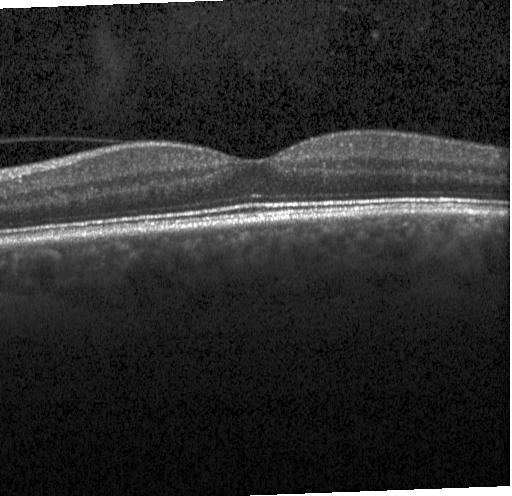 Through the macula; SD-OCT; Heidelberg Spectralis; optical coherence tomography scan — Finding: no choroidal neovascularization, no diabetic macular edema, and no drusen.